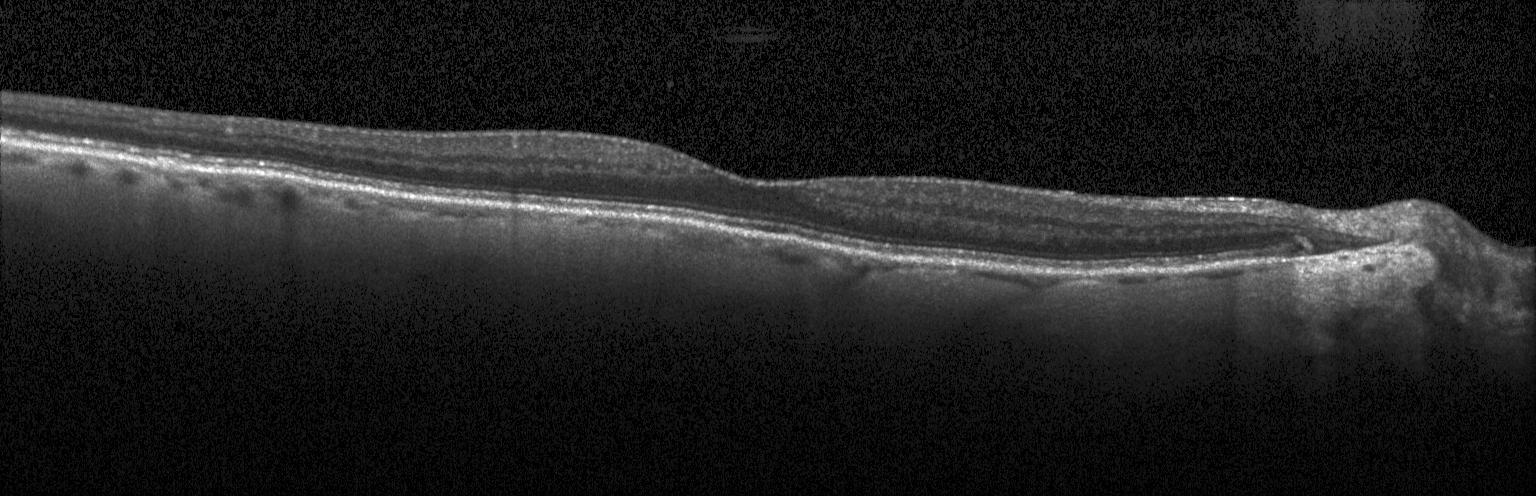

Diagnosis: neither choroidal neovascularization, diabetic macular edema, nor drusen.